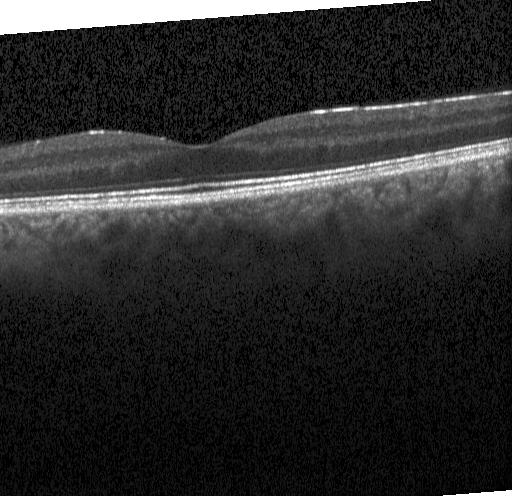

Impression: no choroidal neovascularization, no diabetic macular edema, and no drusen.